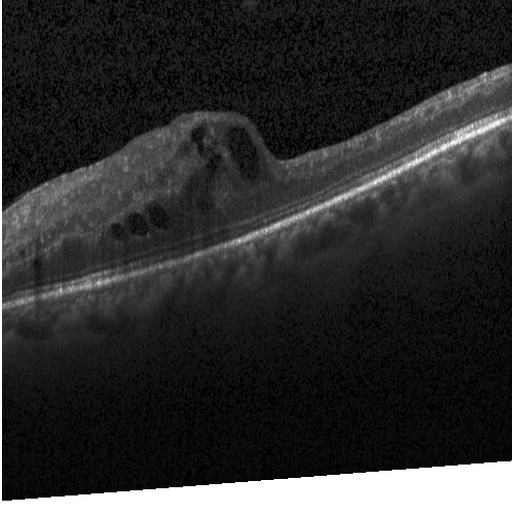
Optical coherence tomography B-scan.
The scan shows diabetic macular edema (DME).